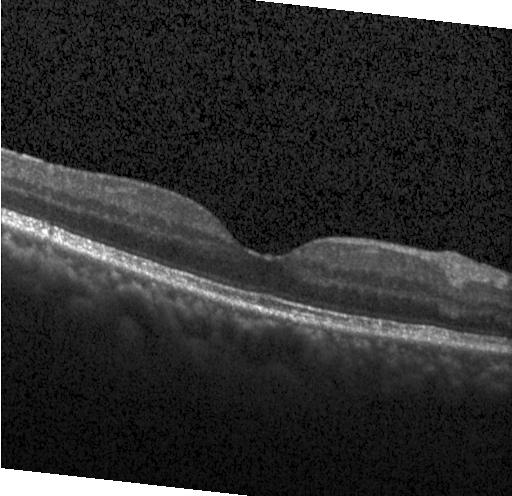

Macular OCT: no choroidal neovascularization, diabetic macular edema, or drusen.